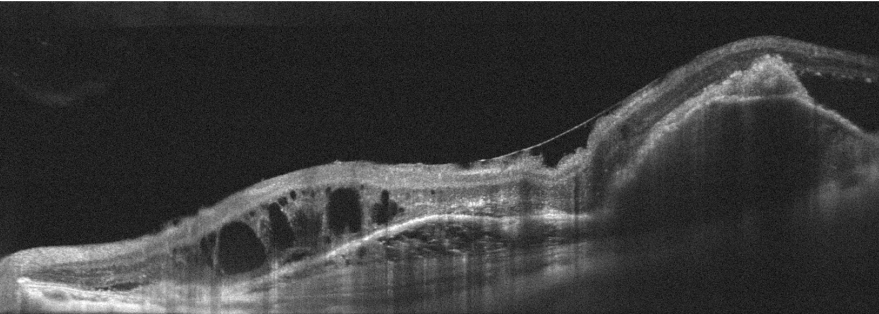

Retinal OCT cross-section, acquired on an Optovue Avanti RTVue XR — Assessment: age-related macular degeneration.